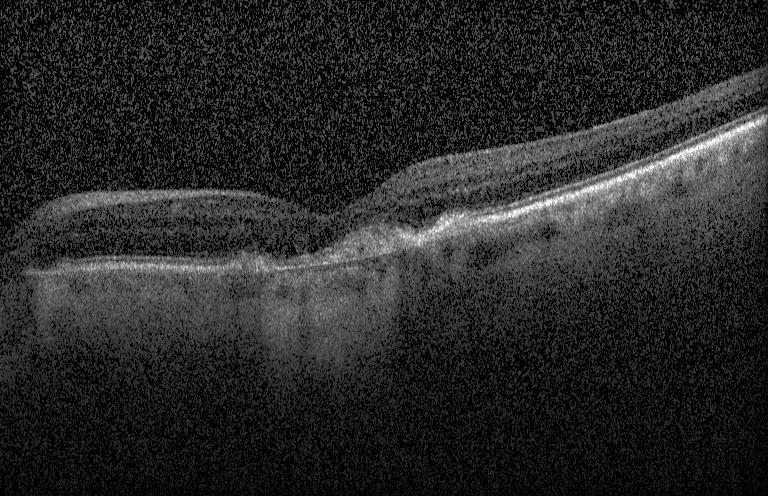
Finding: choroidal neovascularization.